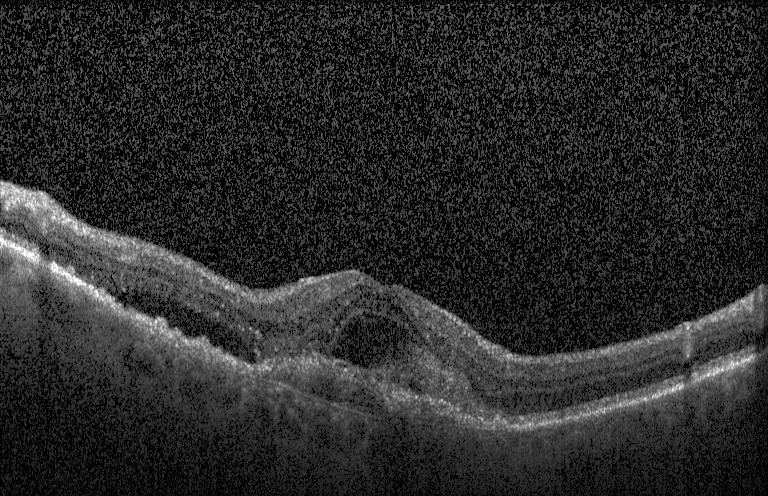

Acquired on a Heidelberg Spectralis; OCT B-scan — Dx: a choroidal neovascular membrane.